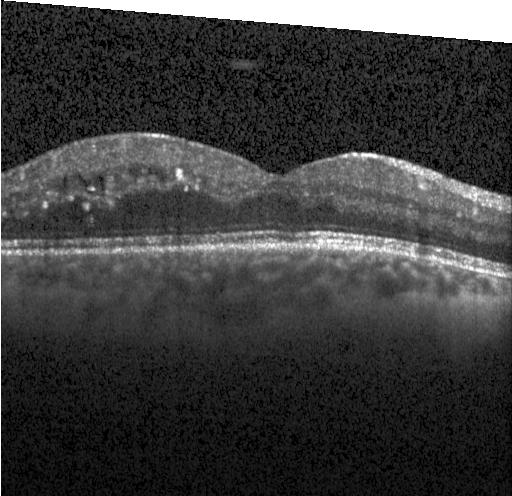
Finding: diabetic macular edema (DME).